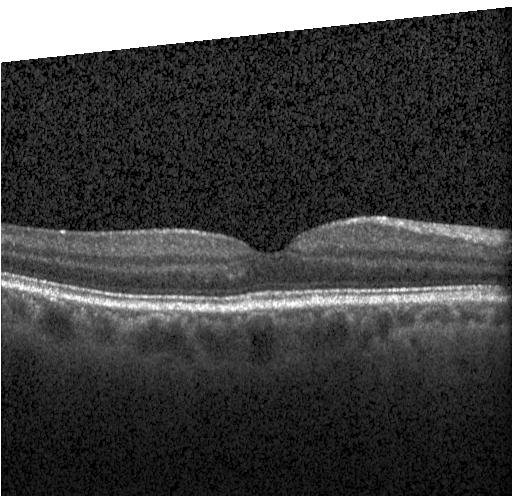 Fovea-centered · spectral-domain optical coherence tomography · OCT line scan · Heidelberg Spectralis OCT system. OCT finding: no choroidal neovascularization, diabetic macular edema, or drusen.